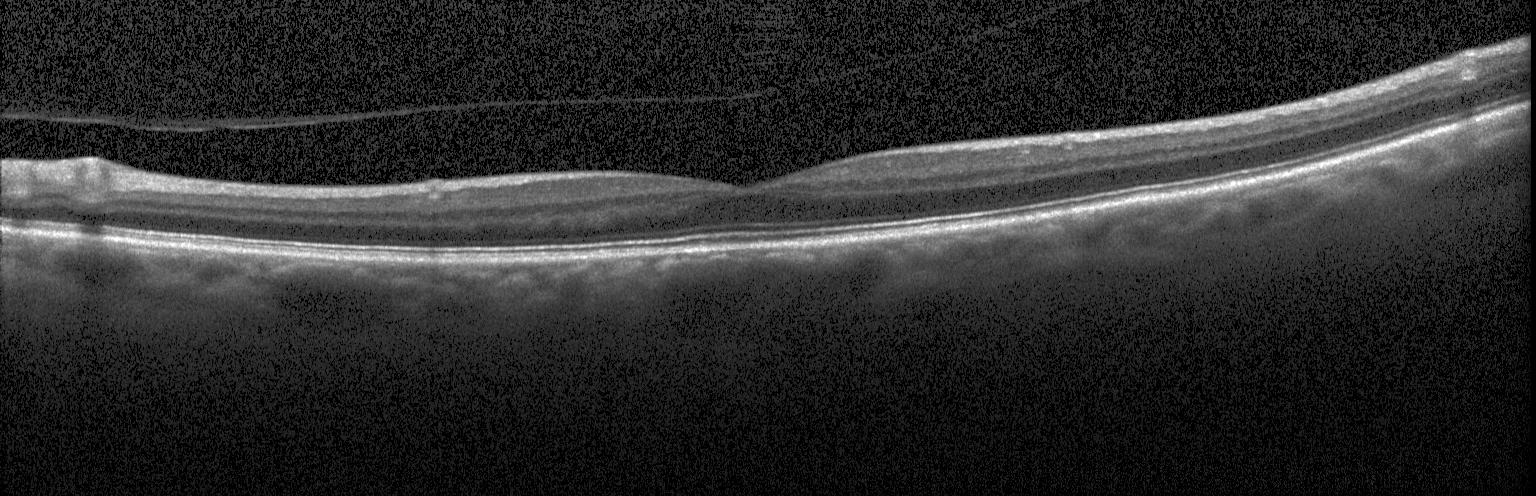

Through the macula, SD-OCT, OCT B-scan, Heidelberg Spectralis. The scan shows no CNV, DME, or drusen.